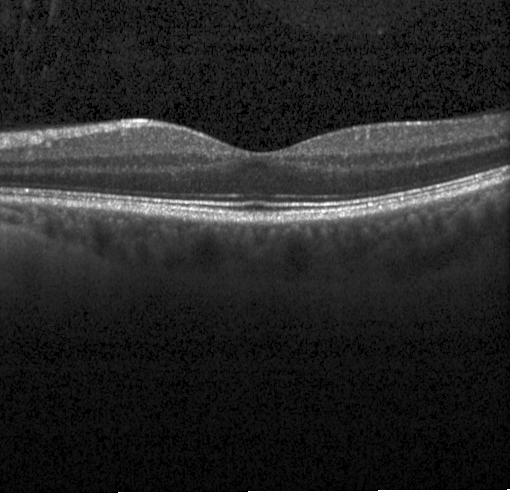
This B-scan demonstrates no evidence of choroidal neovascularization, diabetic macular edema, or drusen.